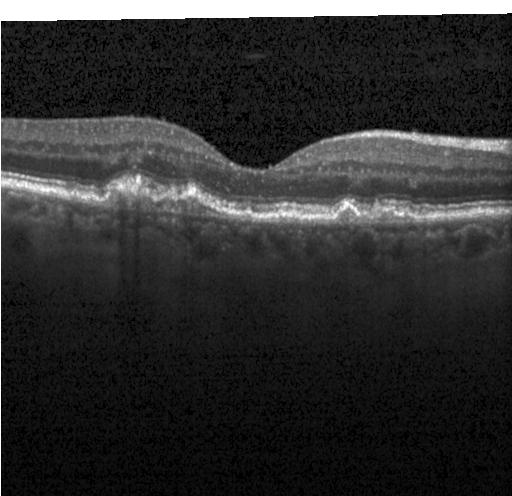

Diagnosis: a choroidal neovascular membrane.